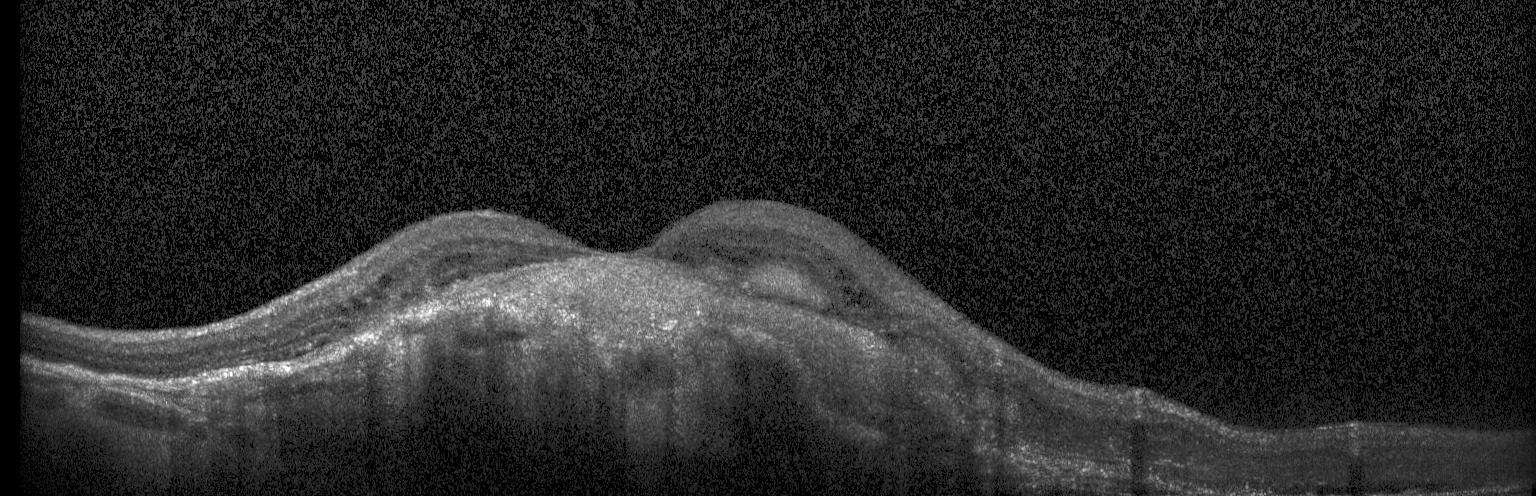

Spectral-domain optical coherence tomography, Heidelberg Spectralis, OCT B-scan
Impression: a choroidal neovascular membrane.